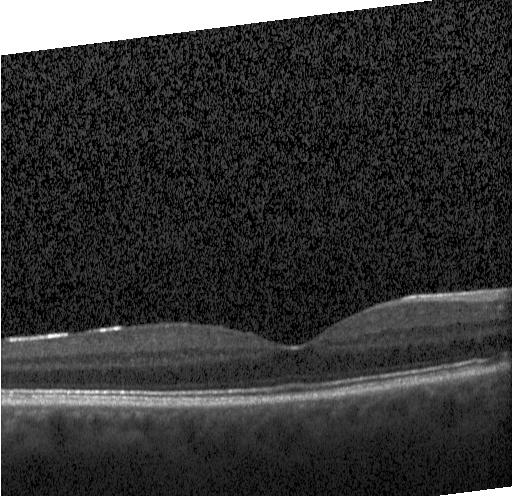

SD-OCT · macular scan · instrument: Heidelberg Spectralis · OCT B-scan. The scan shows neither choroidal neovascularization, diabetic macular edema, nor drusen.